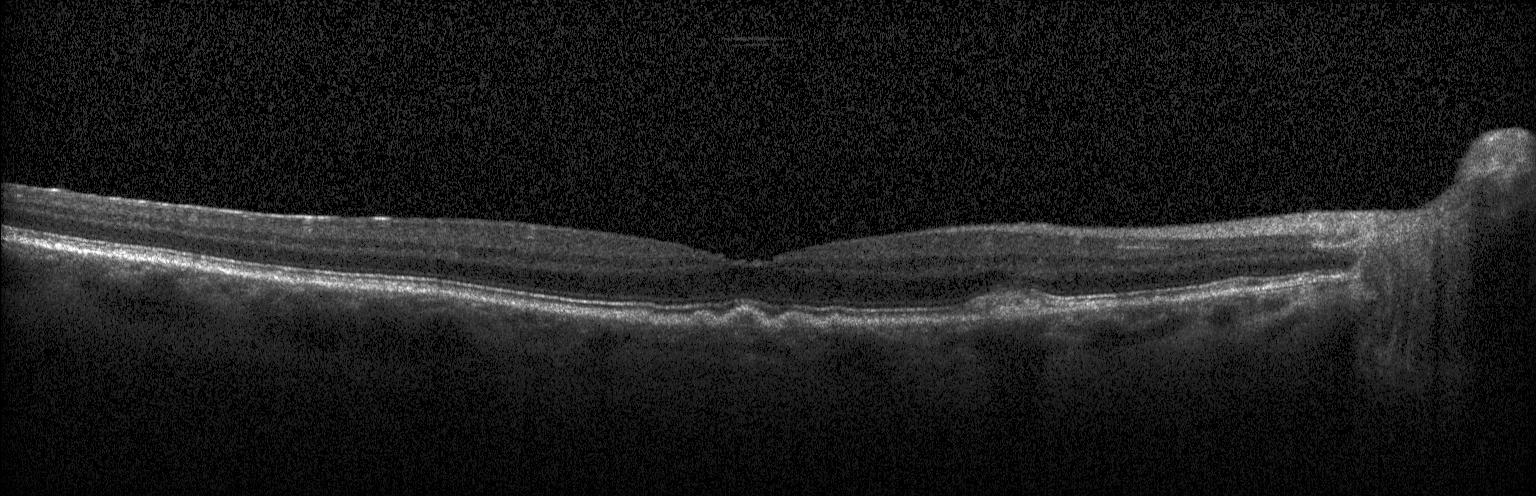 Finding: sub-RPE drusenoid deposits.